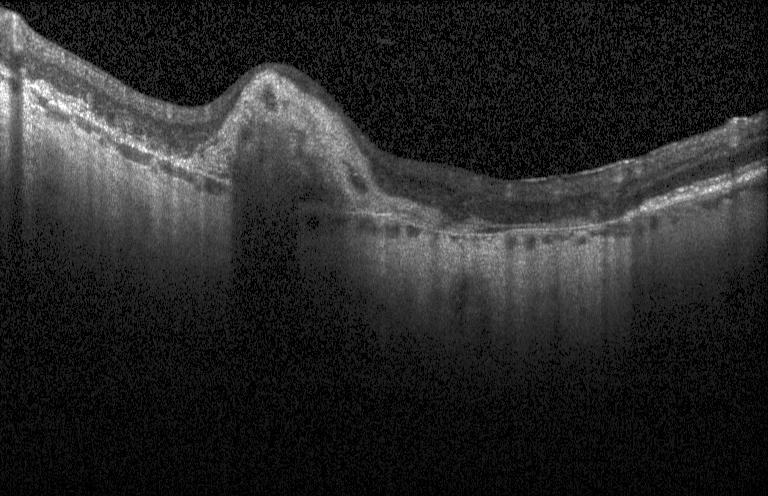

Instrument: Heidelberg Spectralis, optical coherence tomography scan
A choroidal neovascular membrane.